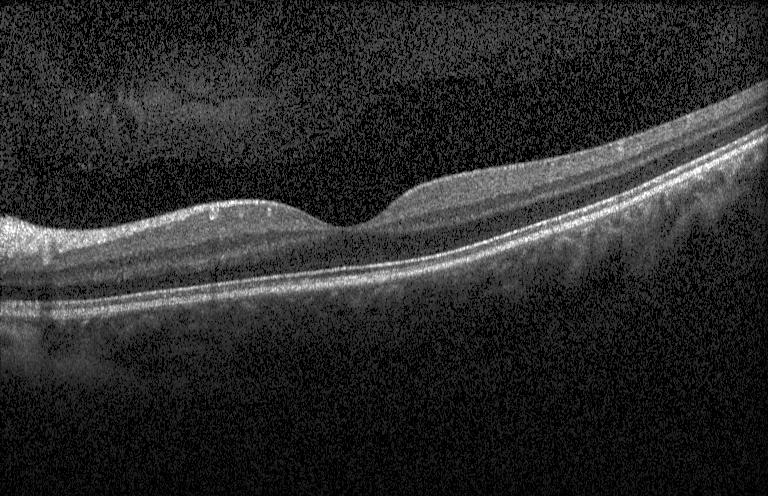 Retinal OCT B-scan; spectral-domain OCT; horizontal scan through the fovea
Dx: no choroidal neovascularization, no diabetic macular edema, and no drusen.